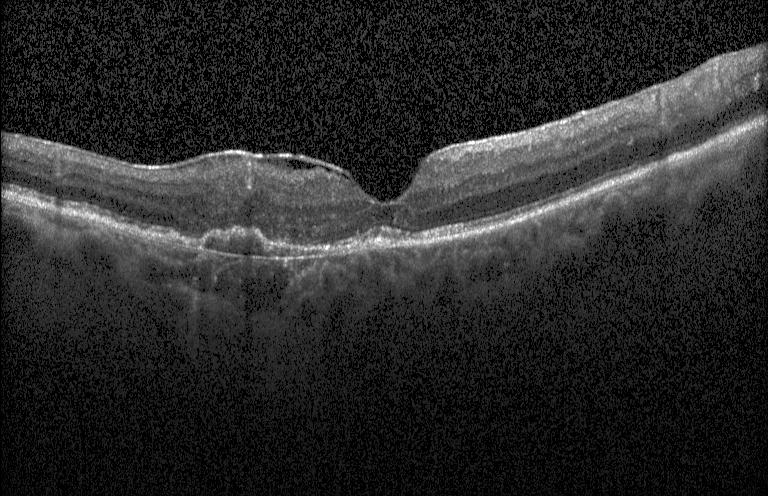 OCT B-scan, macular scan — Impression: a choroidal neovascular membrane.